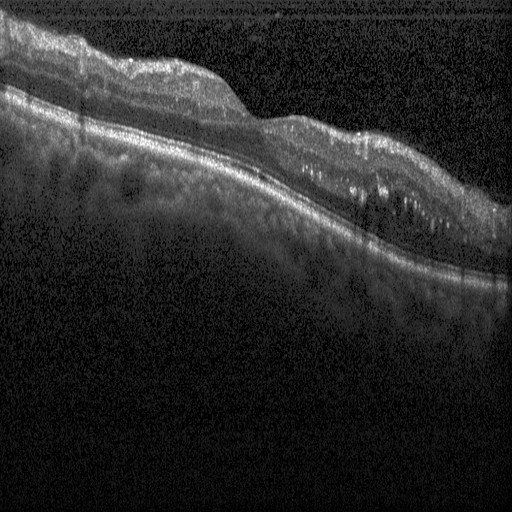 SD-OCT, OCT B-scan. Impression: diabetic macular edema (DME).